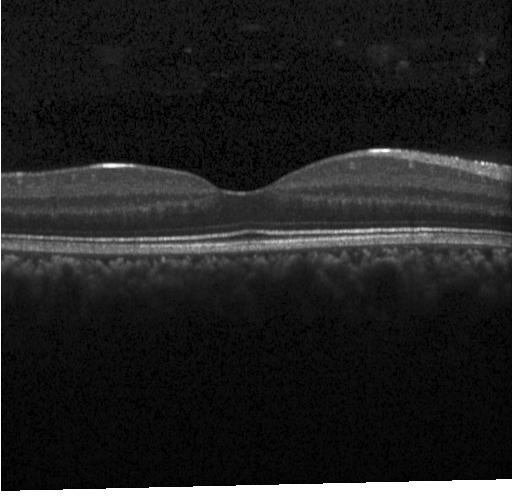
Instrument: Heidelberg Spectralis · spectral-domain optical coherence tomography · centered on the fovea · optical coherence tomography B-scan.
The scan shows no evidence of CNV, DME, or drusen.